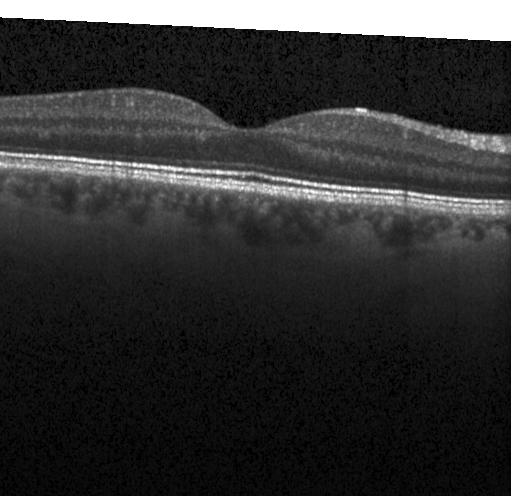
No CNV, DME, or drusen.